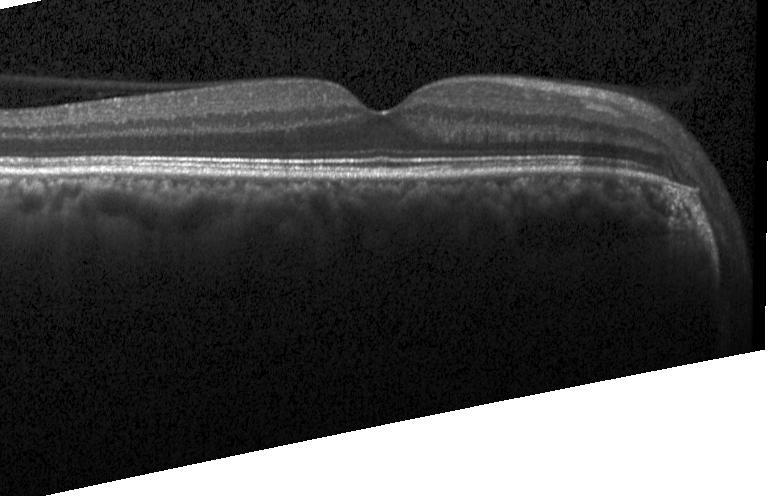

Optical coherence tomography B-scan.
Finding: neither CNV, DME, nor drusen.